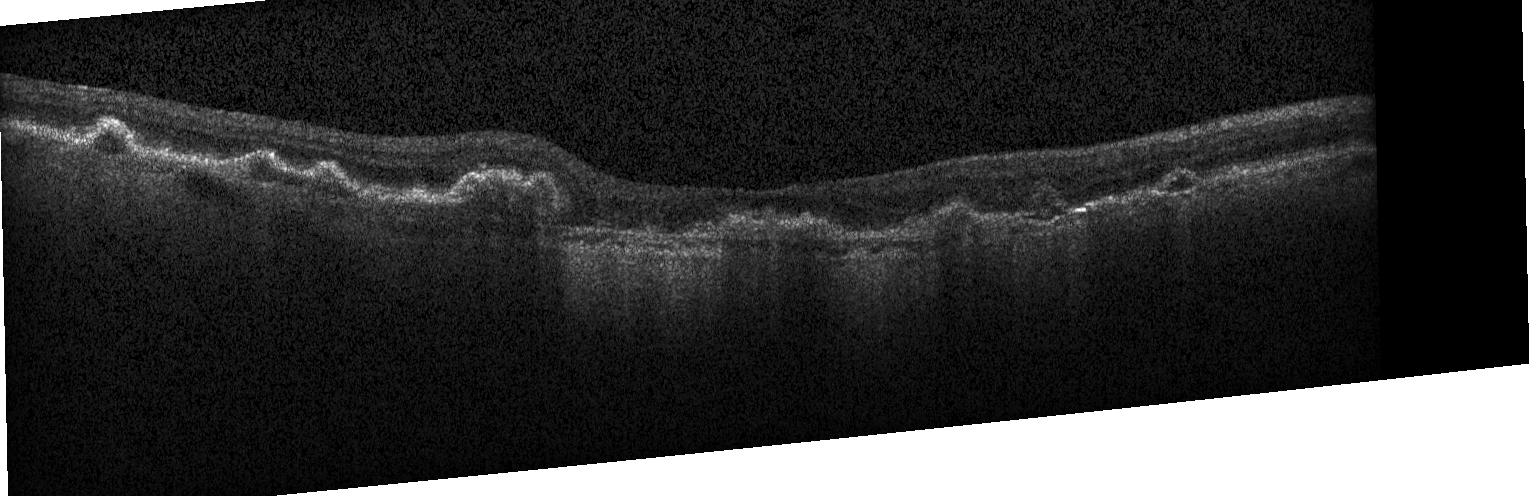
Optical coherence tomography scan. Dx: choroidal neovascularization.